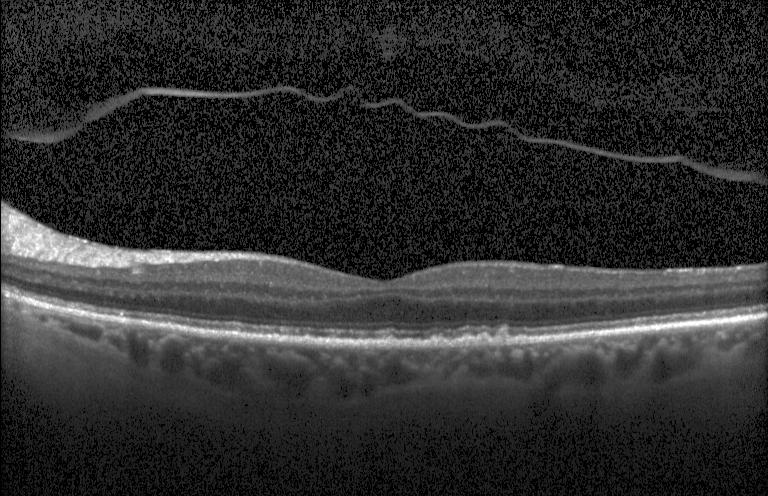
Spectral-domain OCT B-scan: drusen.